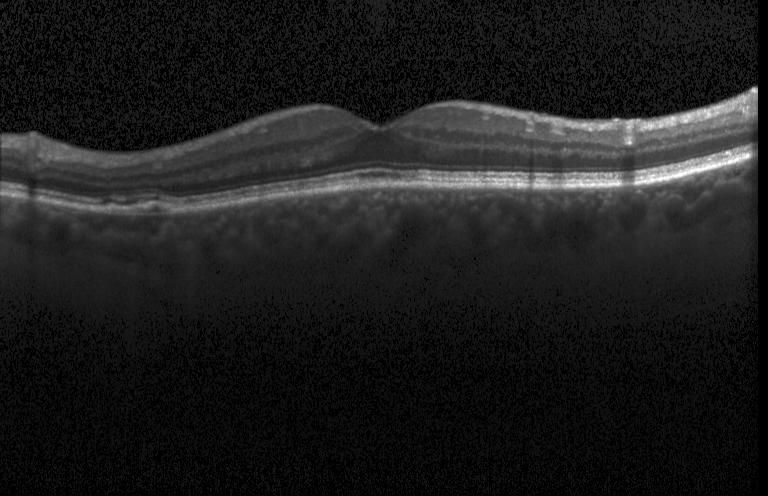 Retinal OCT cross-section. Instrument: Heidelberg Spectralis. SD-OCT. Macular scan — Finding: choroidal neovascularization (CNV).